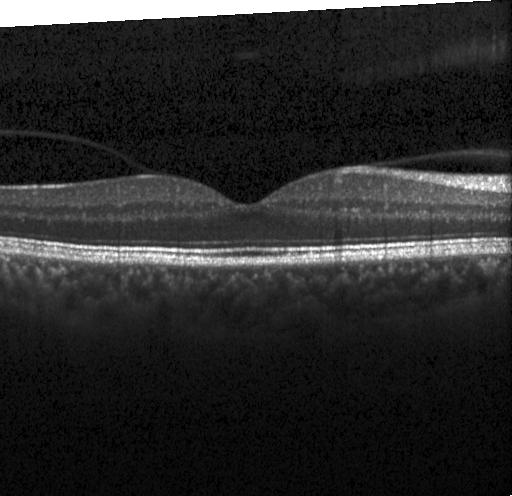
Spectral-domain optical coherence tomography · Heidelberg Spectralis · optical coherence tomography scan. Assessment: no evidence of choroidal neovascularization, diabetic macular edema, or drusen.